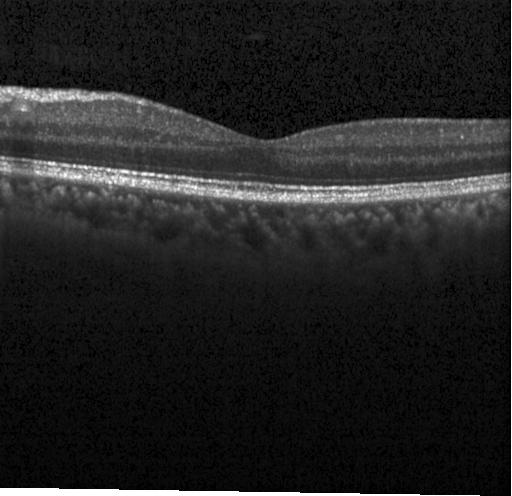

Finding: no evidence of choroidal neovascularization, diabetic macular edema, or drusen.